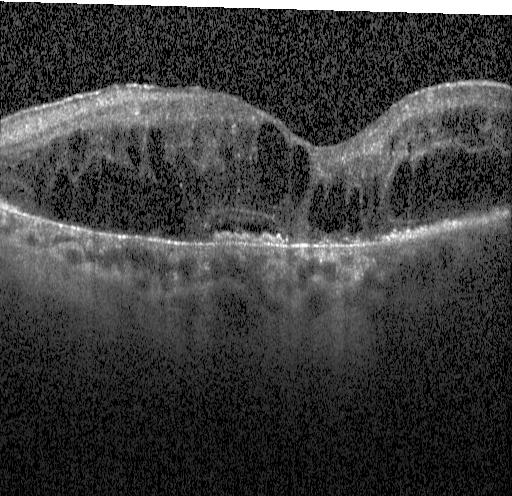

Retinal OCT cross-section; acquired on a Heidelberg Spectralis.
Dx: a choroidal neovascular membrane.